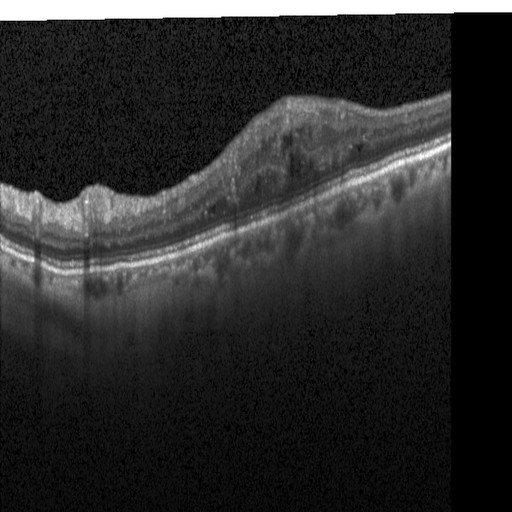

Acquired on a Heidelberg Spectralis; optical coherence tomography B-scan — The scan shows diabetic macular edema (DME).